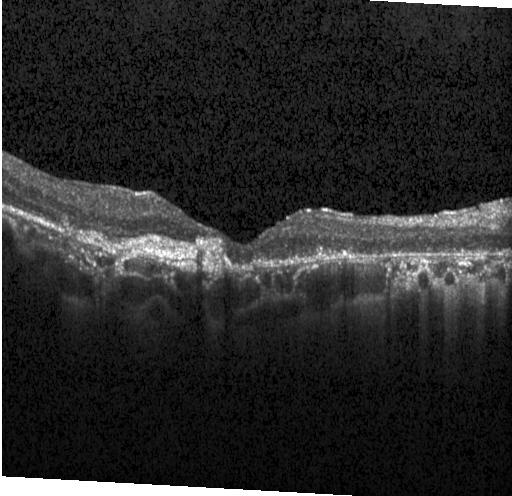 Retinal OCT cross-section showing CNV.